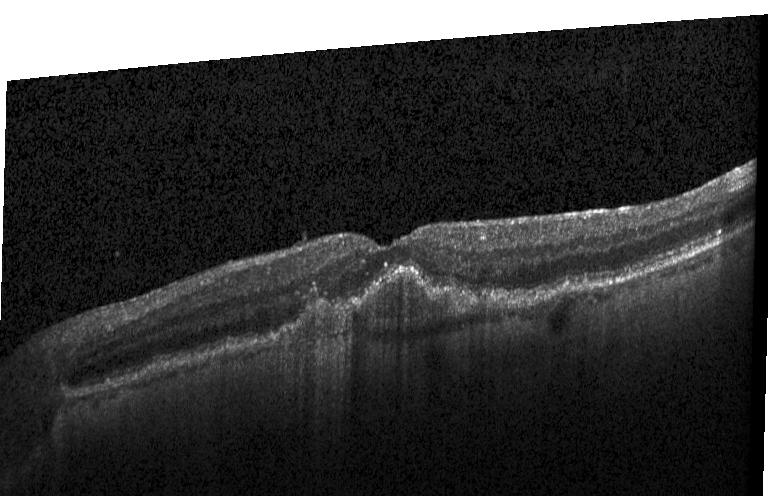 Retinal OCT B-scan — Assessment: a choroidal neovascular membrane.